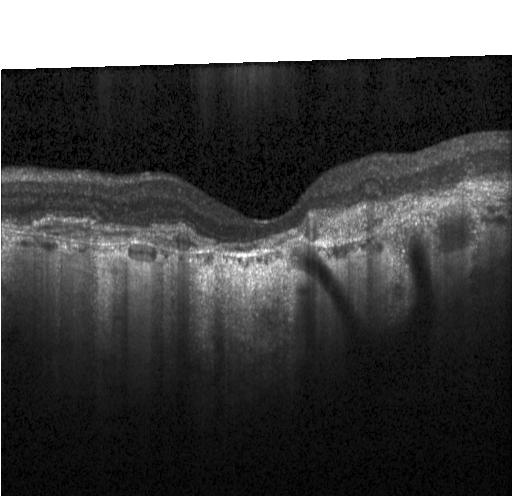

Diagnosis: a choroidal neovascular membrane.